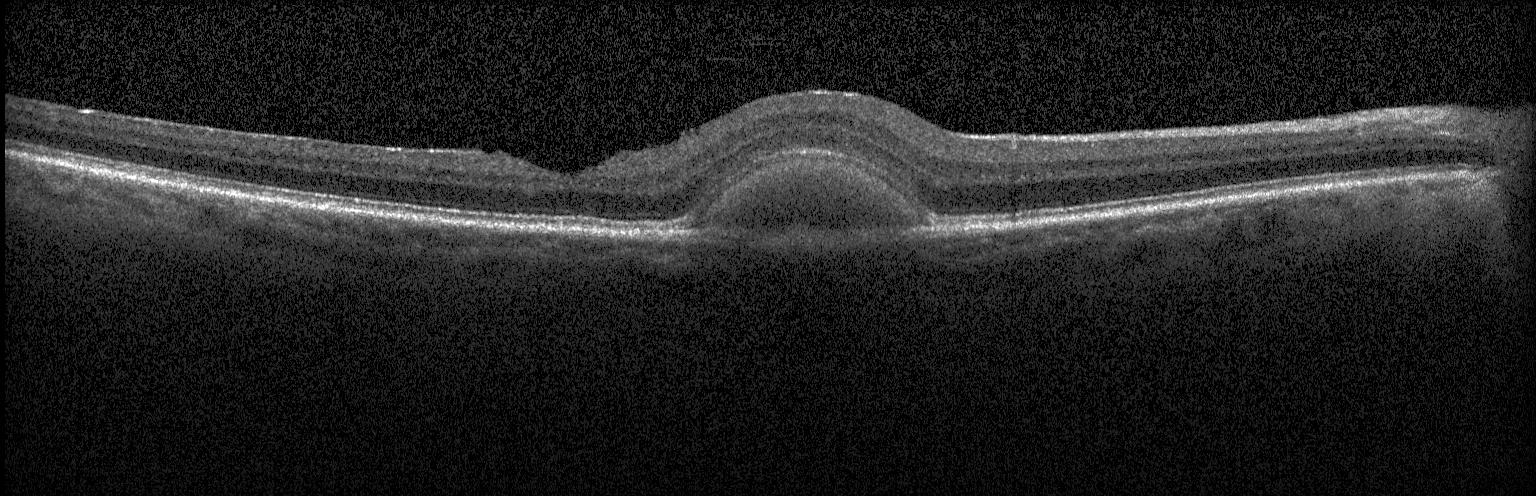
Retinal OCT cross-section — The scan shows CNV.